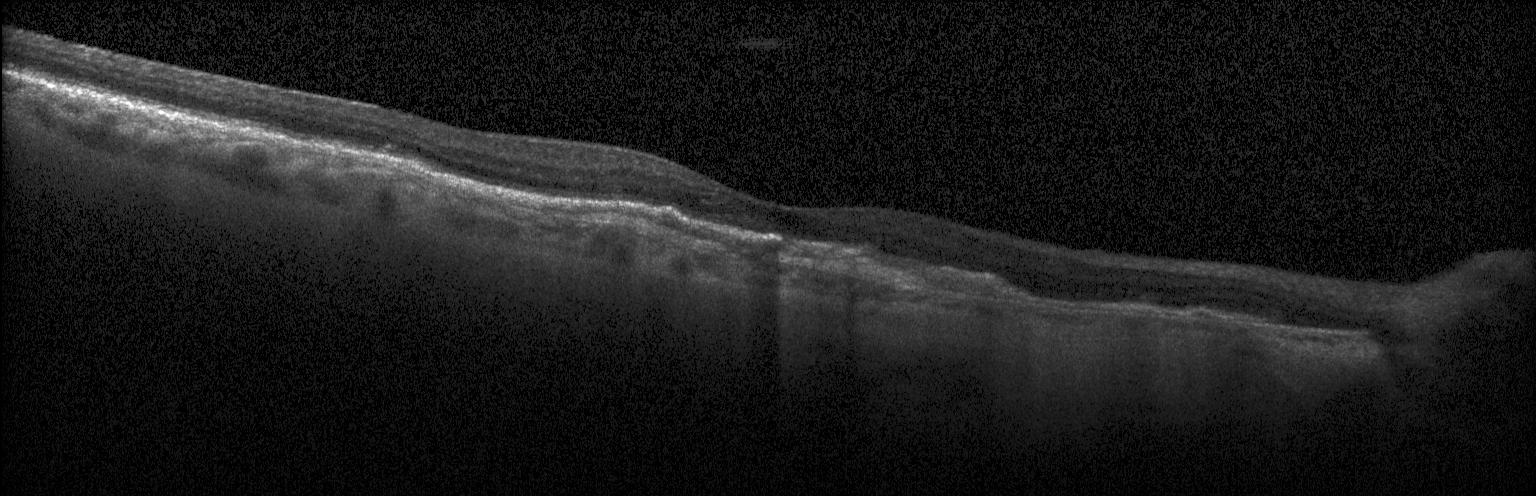
Optical coherence tomography B-scan · Heidelberg Spectralis OCT system · macular scan · SD-OCT. CNV.